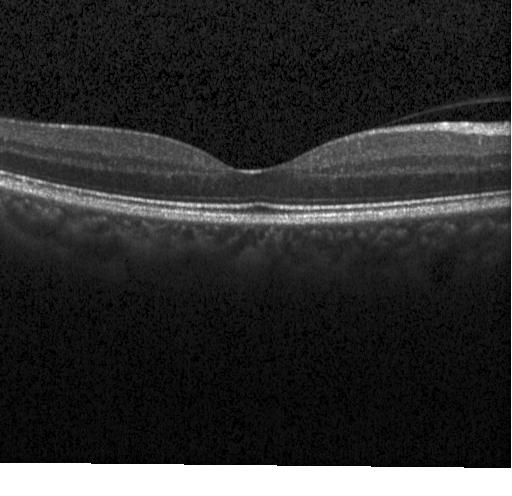 Finding: no choroidal neovascularization, diabetic macular edema, or drusen.